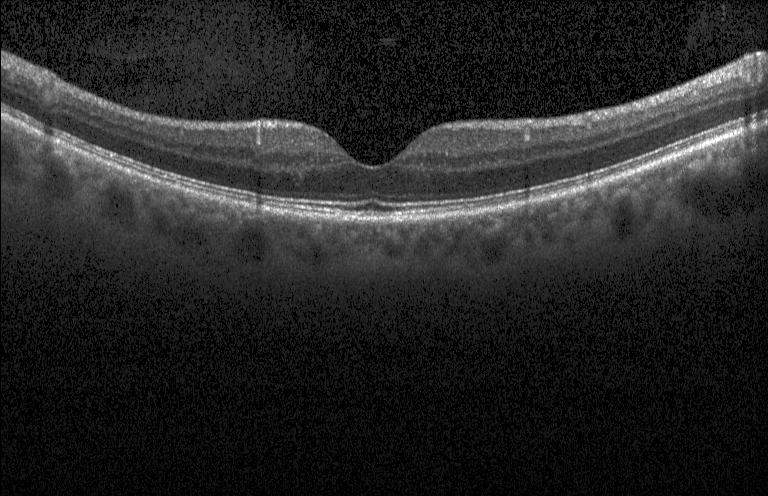

OCT finding: no evidence of choroidal neovascularization, diabetic macular edema, or drusen.